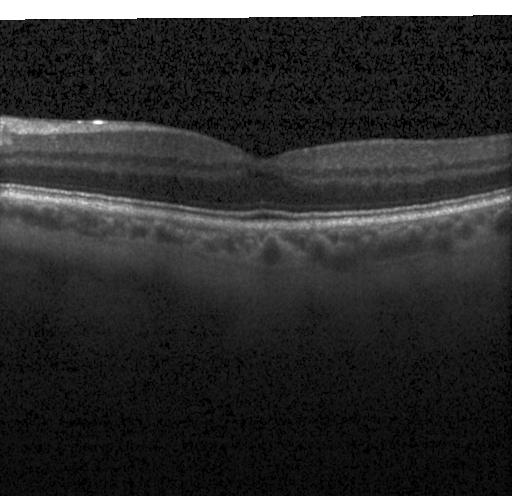 Retinal OCT B-scan; macular scan; SD-OCT — Diagnosis: no choroidal neovascularization, diabetic macular edema, or drusen.